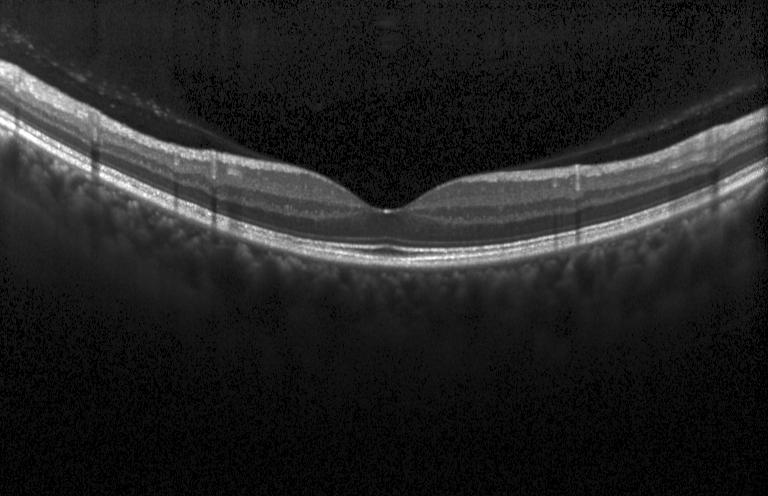 Optical coherence tomography scan; Heidelberg Spectralis OCT system; through the macula; spectral-domain OCT — Impression: no choroidal neovascularization, no diabetic macular edema, and no drusen.